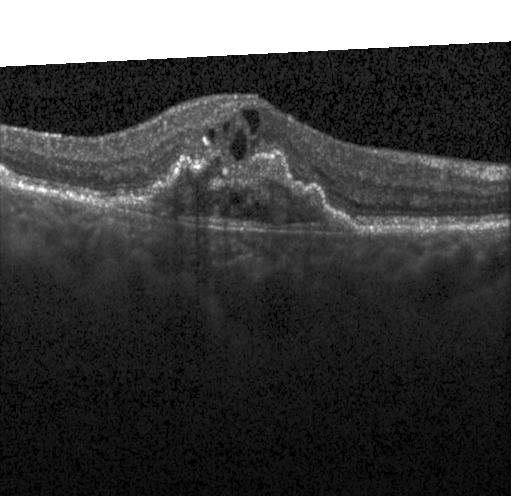 Instrument: Heidelberg Spectralis · centered on the fovea · OCT line scan. This B-scan demonstrates a choroidal neovascular membrane.